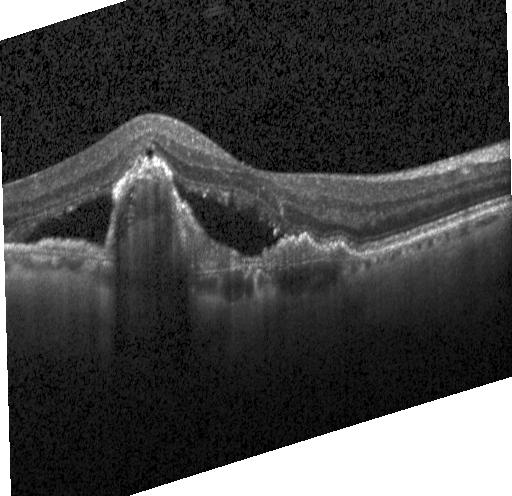 Choroidal neovascularization (CNV).